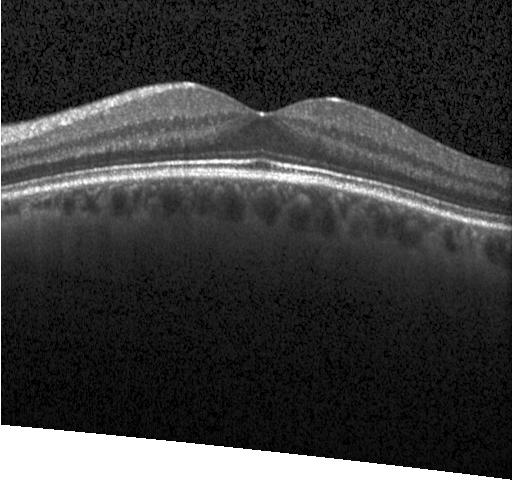 Impression: no evidence of choroidal neovascularization, diabetic macular edema, or drusen.